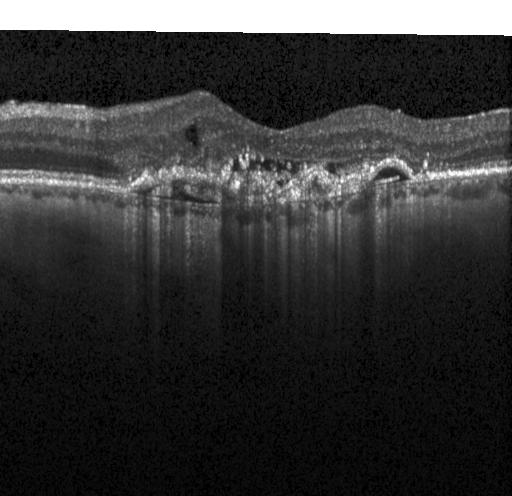
SD-OCT, retinal OCT B-scan. Assessment: choroidal neovascularization.